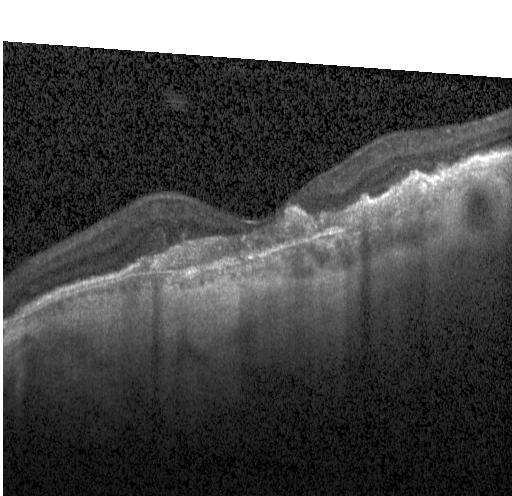 OCT line scan. Macular scan. Heidelberg Spectralis. Spectral-domain optical coherence tomography — Finding: choroidal neovascularization (CNV).